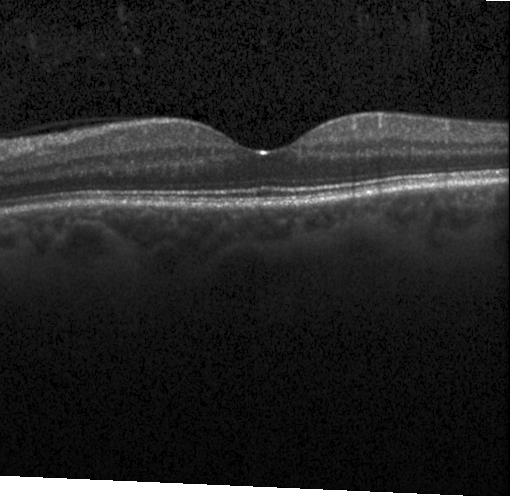
Optical coherence tomography B-scan; instrument: Heidelberg Spectralis; through the macula
Dx: no evidence of choroidal neovascularization, diabetic macular edema, or drusen.